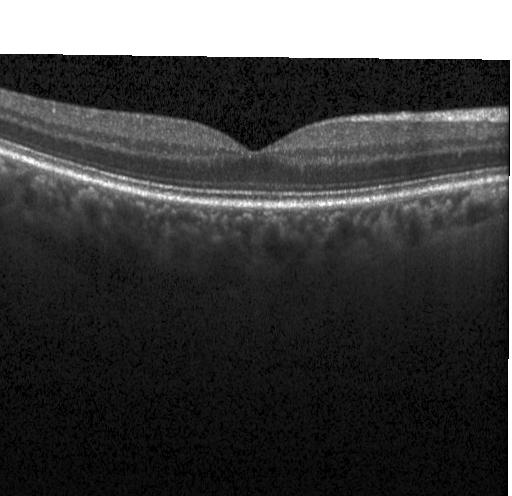 Macular scan; Heidelberg Spectralis; OCT B-scan — Diagnosis: no choroidal neovascularization, diabetic macular edema, or drusen.